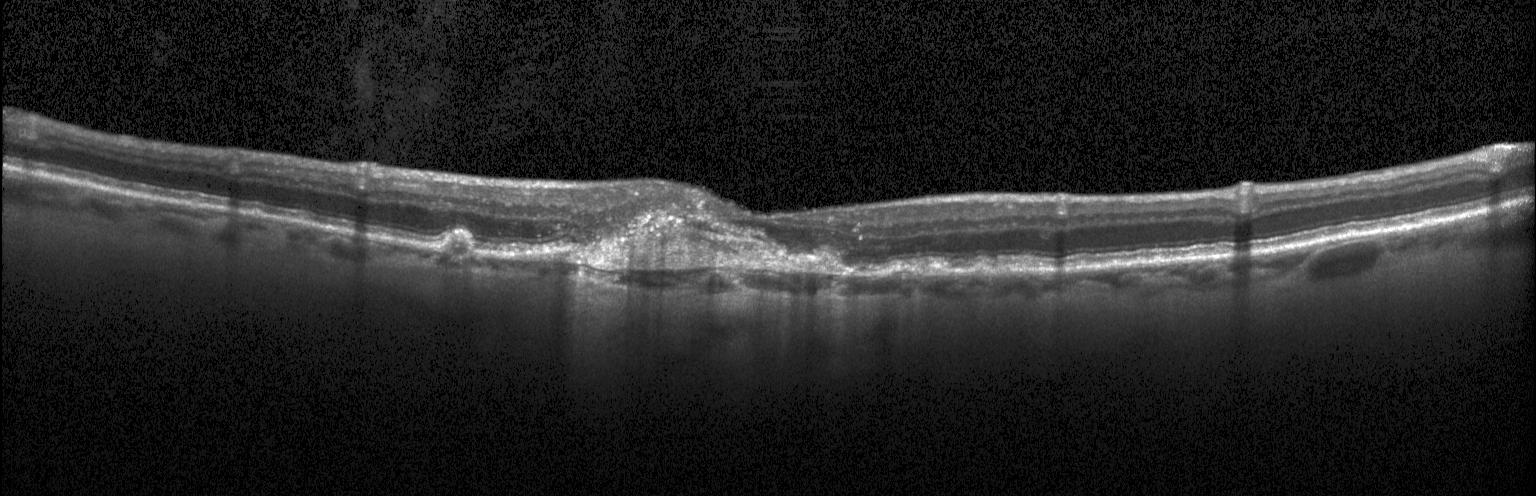 Spectral-domain optical coherence tomography. Heidelberg Spectralis. Retinal OCT B-scan. Fovea-centered
This B-scan demonstrates choroidal neovascularization.